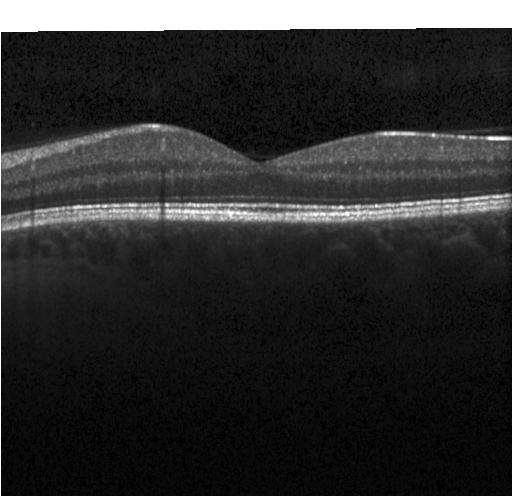

Spectral-domain optical coherence tomography, optical coherence tomography B-scan, macular scan, acquired on a Heidelberg Spectralis — Impression: no choroidal neovascularization, diabetic macular edema, or drusen.